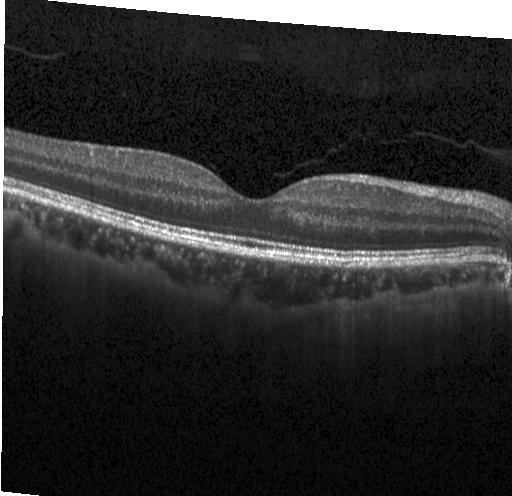 This B-scan demonstrates no choroidal neovascularization, no diabetic macular edema, and no drusen.